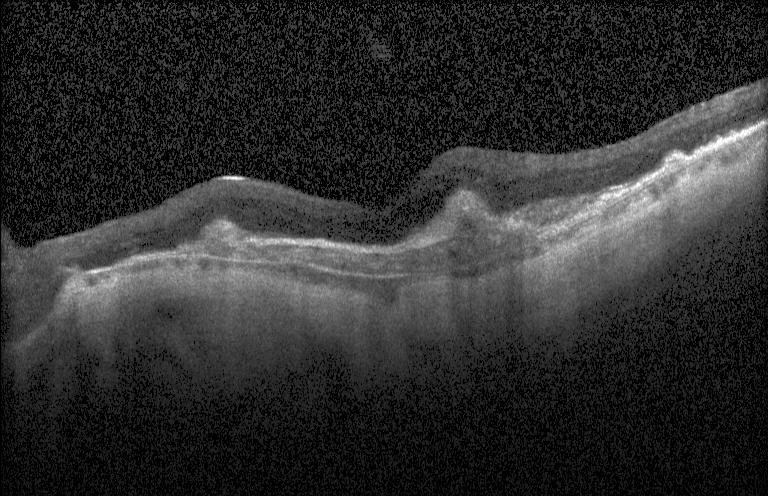

Spectral-domain OCT, retinal OCT B-scan — This B-scan demonstrates choroidal neovascularization (CNV).